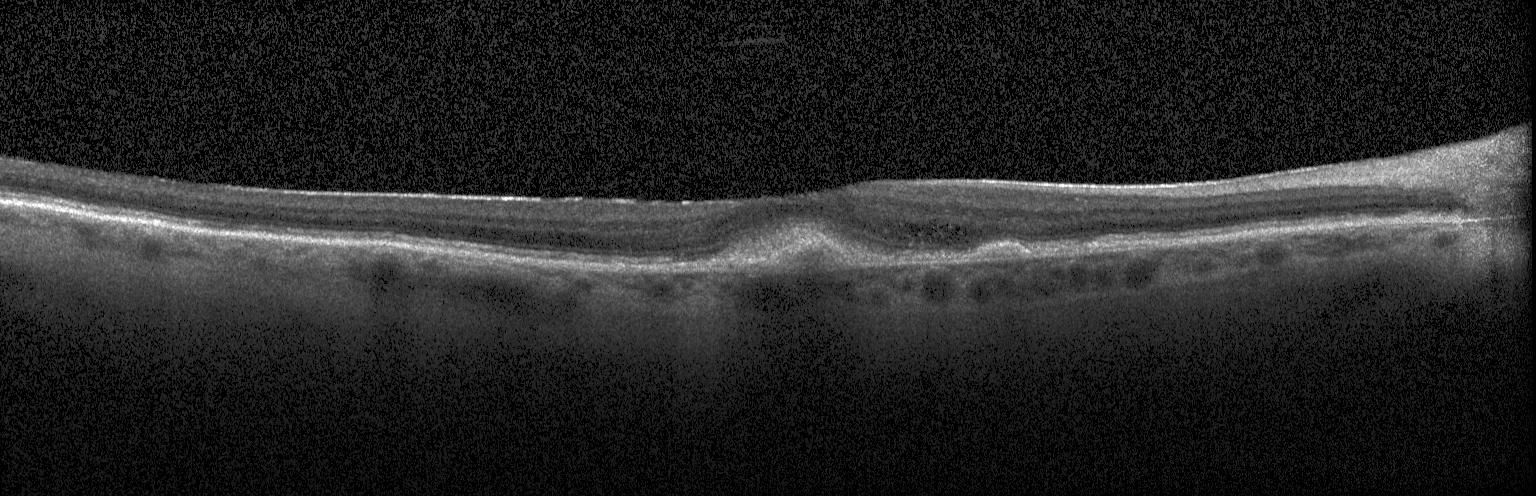
Macular OCT demonstrating choroidal neovascularization (CNV).